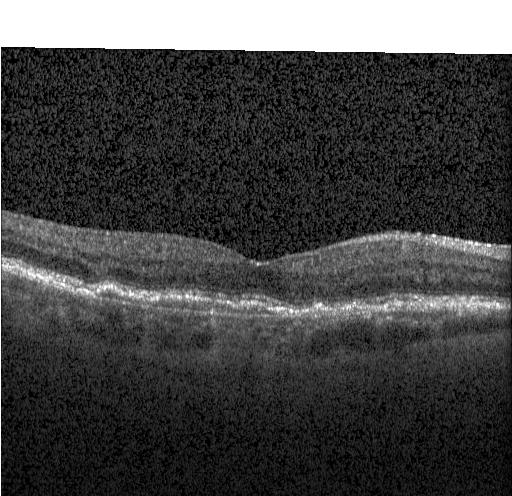
Retinal OCT B-scan. OCT finding: choroidal neovascularization.